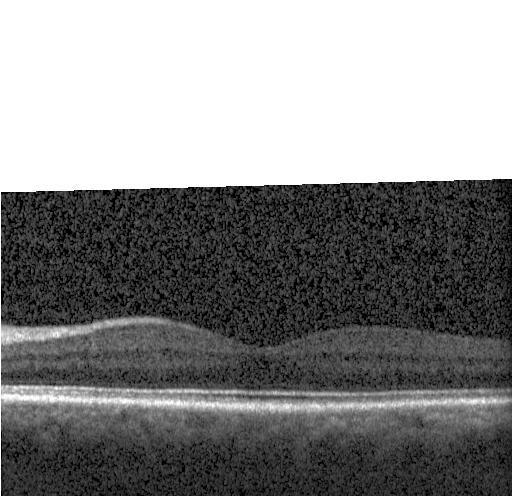
Optical coherence tomography B-scan
This B-scan demonstrates neither CNV, DME, nor drusen.